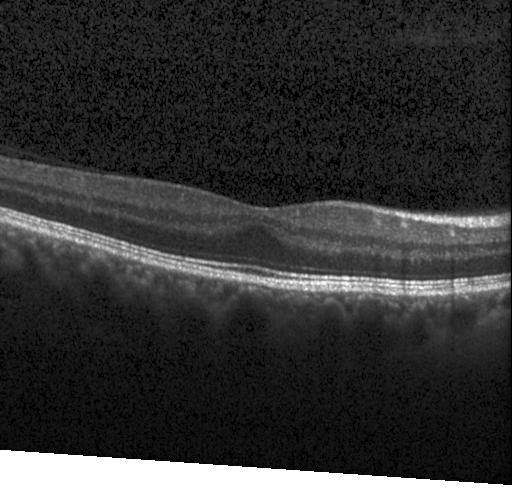
OCT B-scan. Diagnosis: no evidence of CNV, DME, or drusen.